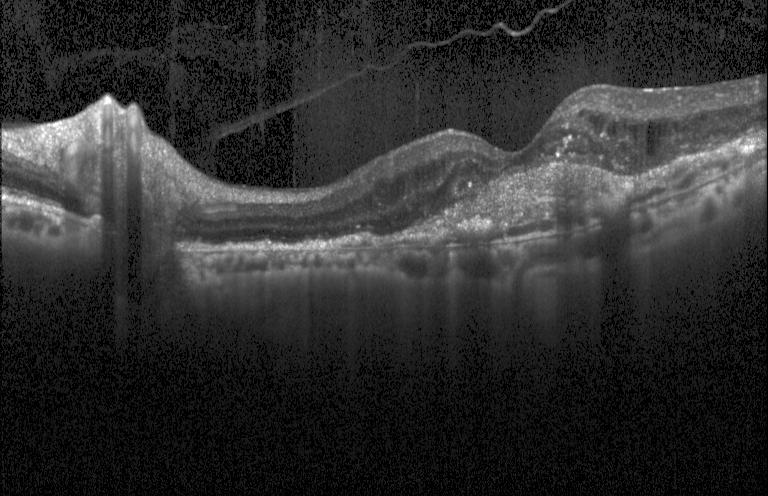

Optical coherence tomography scan. Acquired on a Heidelberg Spectralis.
Macular OCT: CNV.